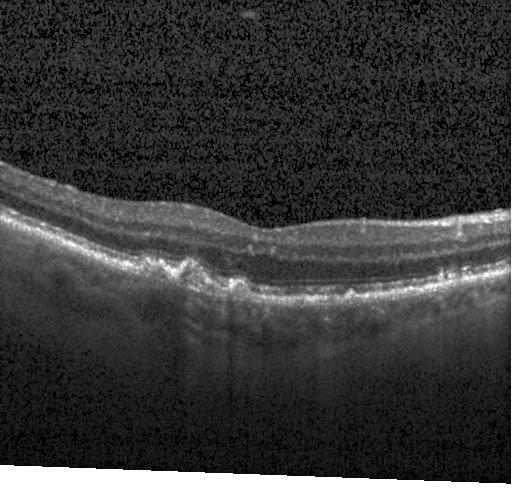 Heidelberg Spectralis, retinal OCT B-scan, through the macula, spectral-domain OCT. Macular OCT: multiple drusen.